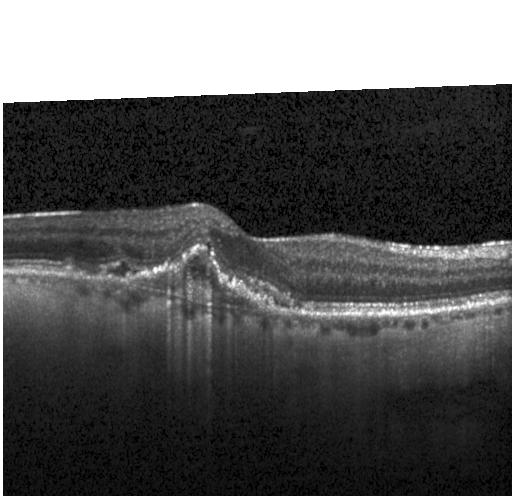 OCT finding: CNV.